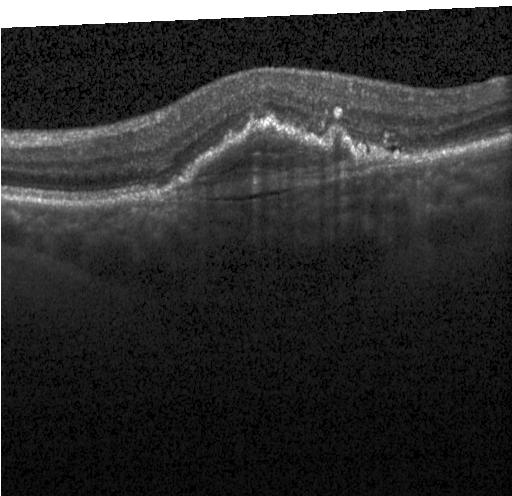 Diagnosis: choroidal neovascularization.